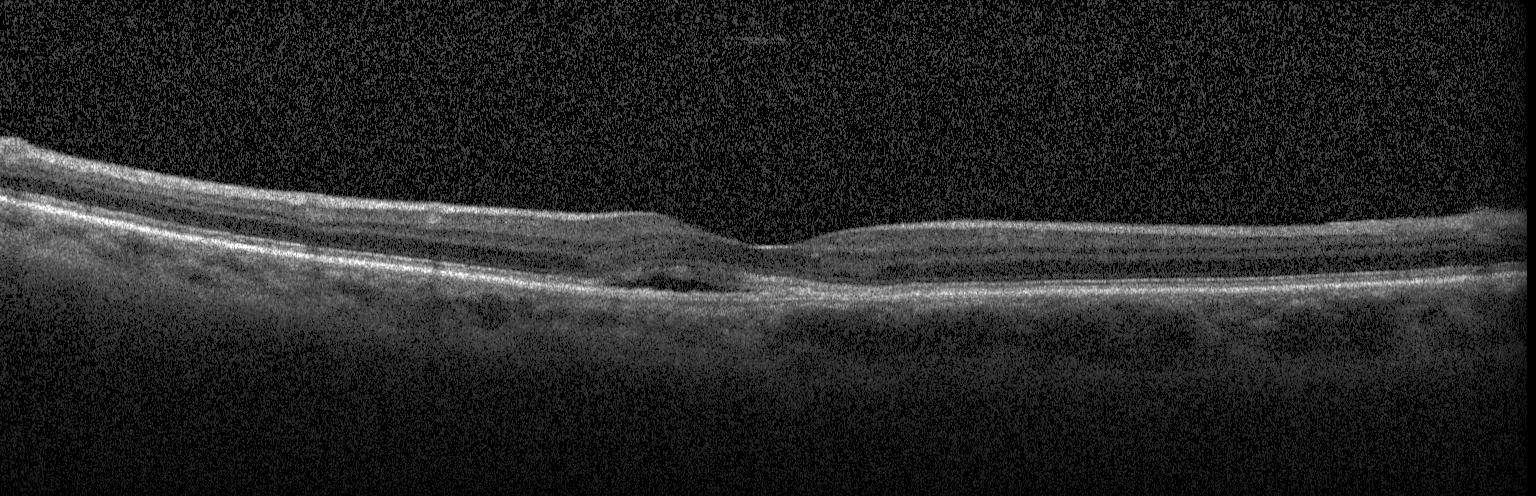 Spectral-domain optical coherence tomography; optical coherence tomography B-scan
Impression: a choroidal neovascular membrane.